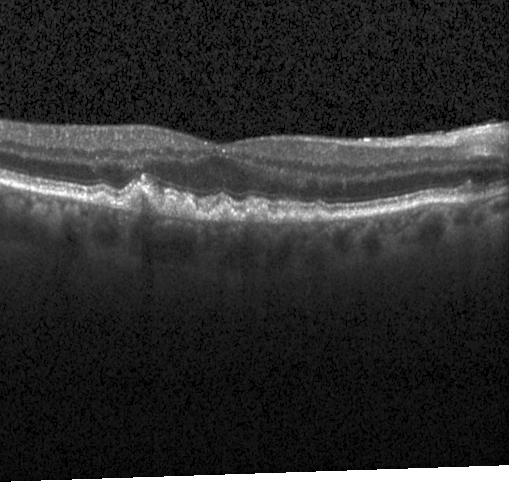 Retinal OCT B-scan · Heidelberg Spectralis · spectral-domain OCT. Multiple drusen.